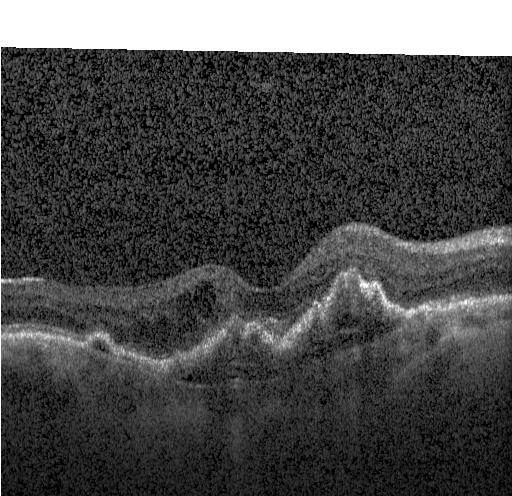
Choroidal neovascularization (CNV).